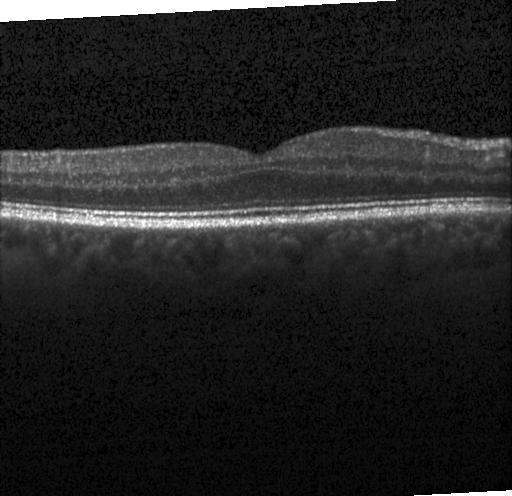

Retinal OCT B-scan.
Macular OCT: no choroidal neovascularization, no diabetic macular edema, and no drusen.